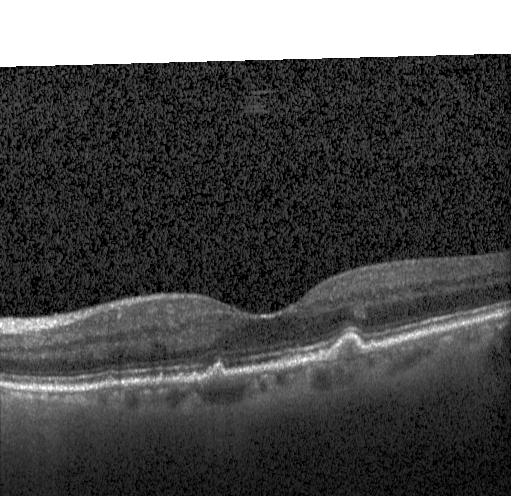

Macular OCT demonstrating sub-RPE drusenoid deposits.